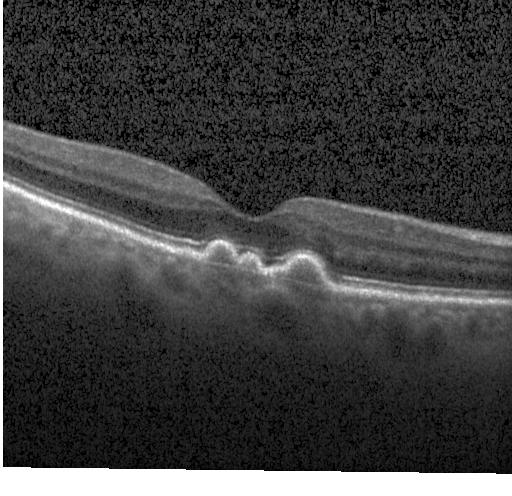
This B-scan demonstrates multiple drusen.